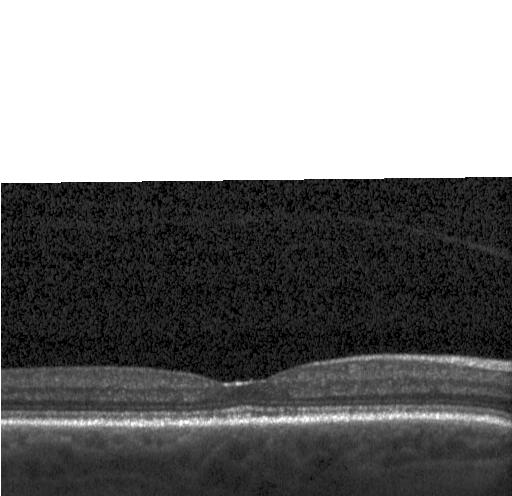

Macular scan. Optical coherence tomography scan.
Dx: no choroidal neovascularization, no diabetic macular edema, and no drusen.